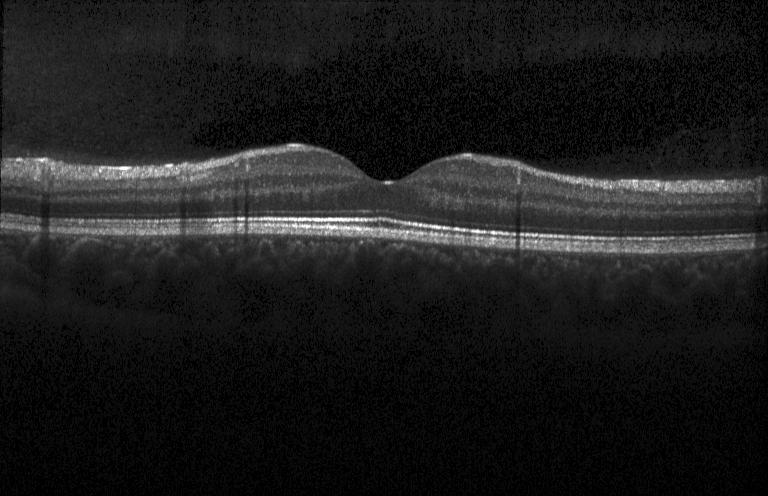 Heidelberg Spectralis, OCT B-scan, SD-OCT.
The scan shows no CNV, no DME, and no drusen.